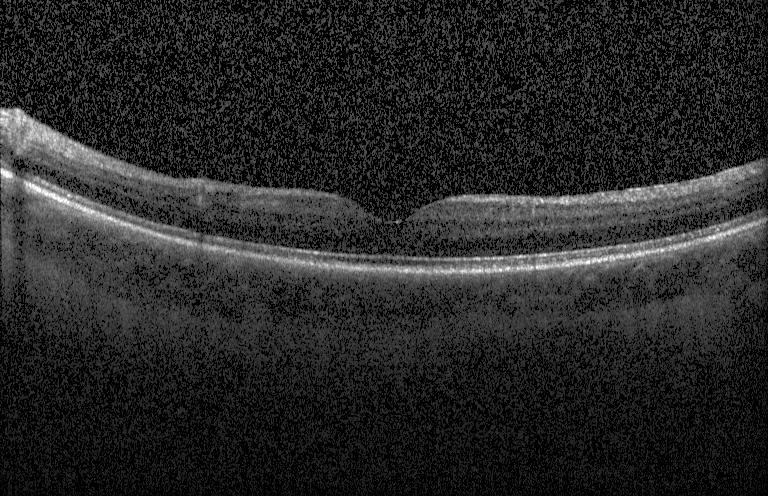
Fovea-centered, Heidelberg Spectralis, retinal OCT cross-section. OCT finding: no choroidal neovascularization, diabetic macular edema, or drusen.